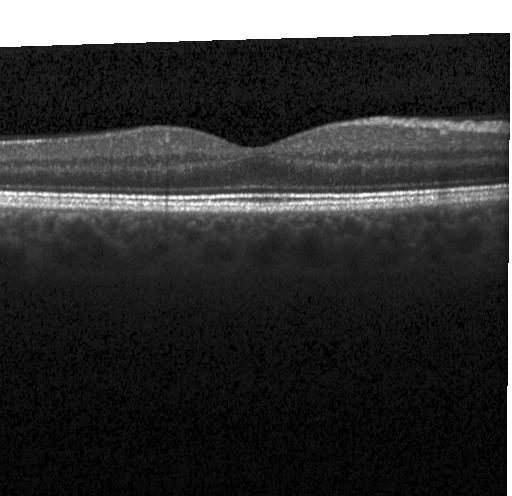
Spectral-domain optical coherence tomography; horizontal scan through the fovea; retinal OCT cross-section.
The scan shows no choroidal neovascularization, no diabetic macular edema, and no drusen.